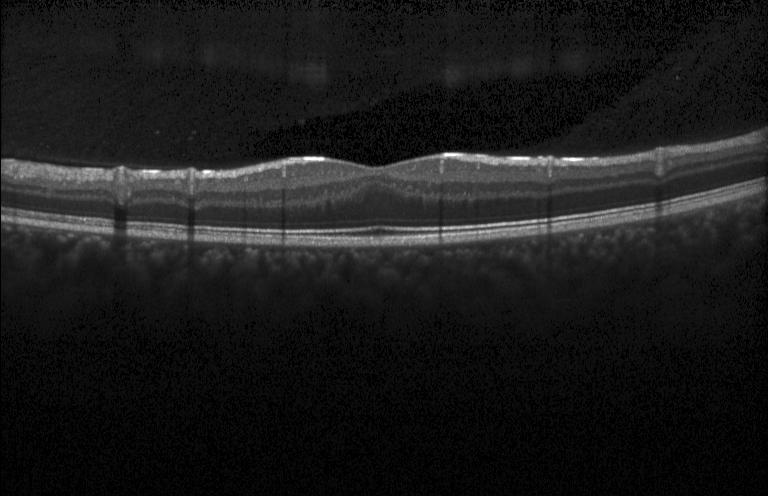

Acquired on a Heidelberg Spectralis. Horizontal scan through the fovea. Spectral-domain OCT. Optical coherence tomography scan — This B-scan demonstrates no choroidal neovascularization, diabetic macular edema, or drusen.